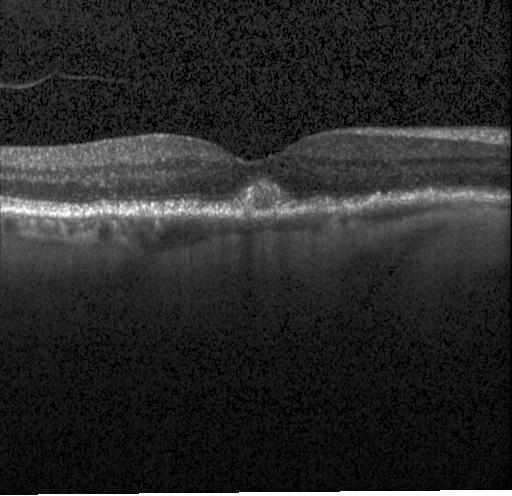 Optical coherence tomography scan, spectral-domain OCT, Heidelberg Spectralis, fovea-centered
Diagnosis: sub-RPE drusenoid deposits.